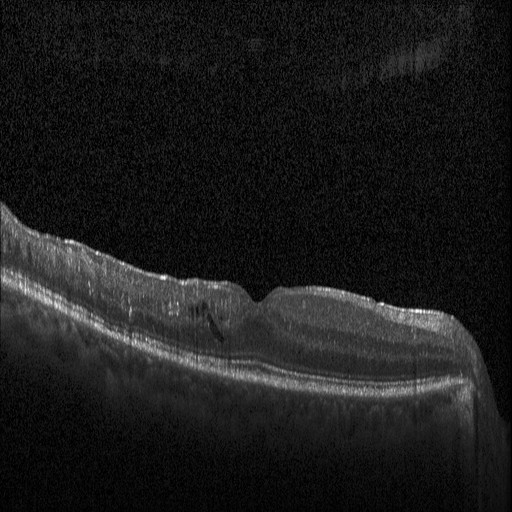
Impression: diabetic macular edema (DME).